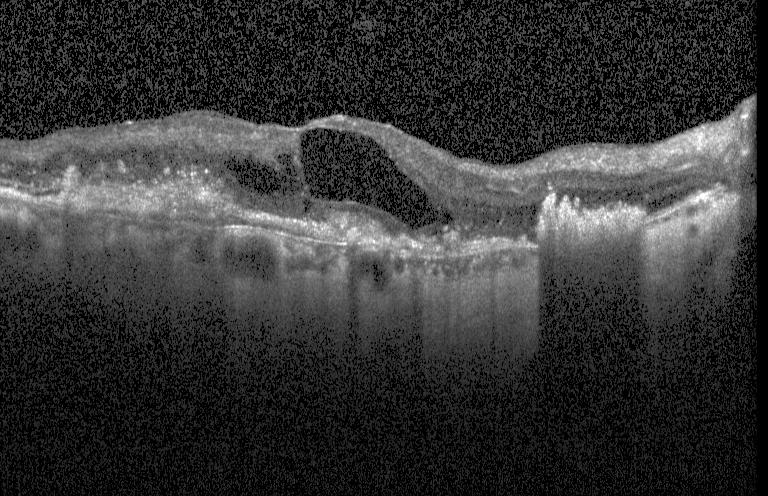
Diagnosis: CNV.